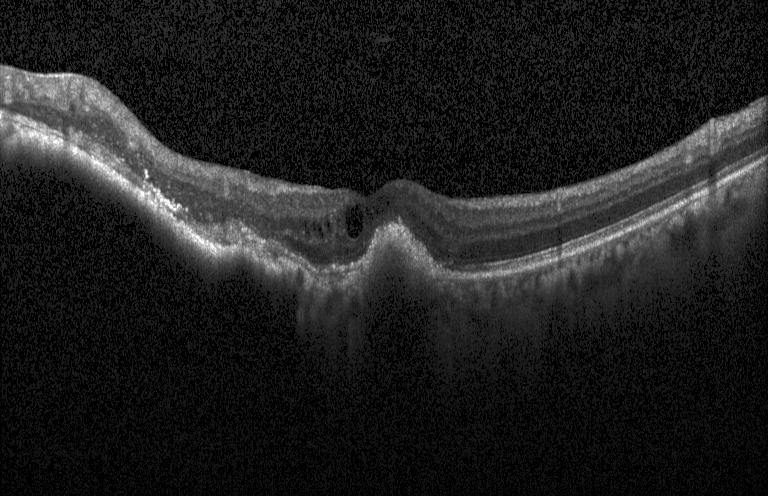

Diagnosis: a choroidal neovascular membrane.